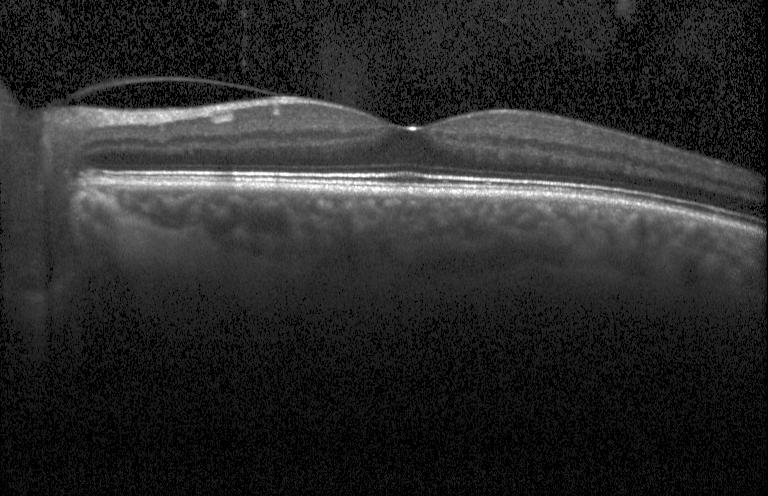
Finding: no evidence of choroidal neovascularization, diabetic macular edema, or drusen.